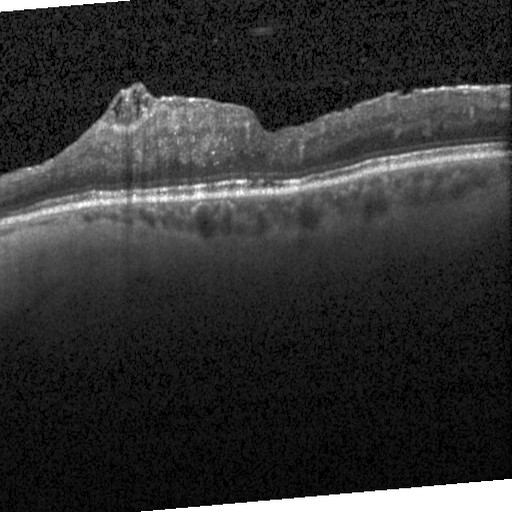
Macular OCT: diabetic macular edema (DME).